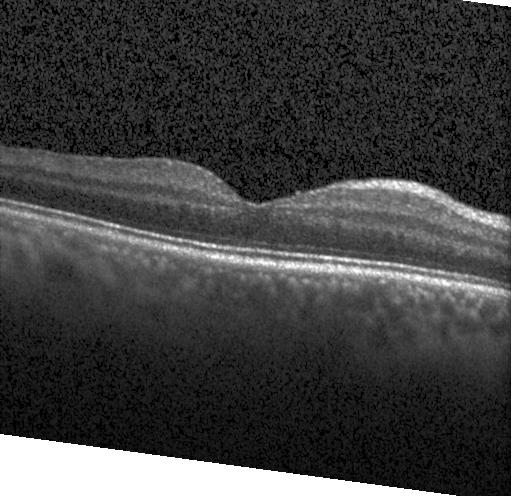

Retinal OCT cross-section — Finding: no choroidal neovascularization, diabetic macular edema, or drusen.